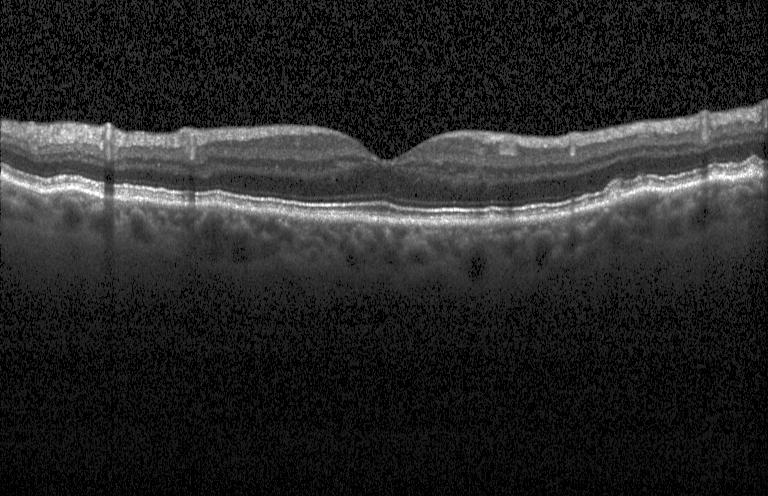

Acquired on a Heidelberg Spectralis · through the macula · spectral-domain OCT · retinal OCT cross-section — Diagnosis: drusen.